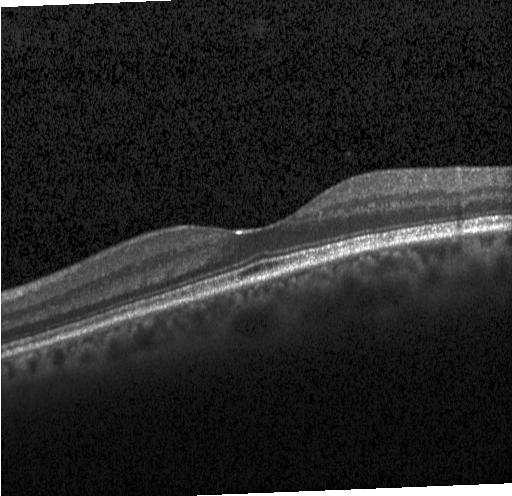

Finding: no choroidal neovascularization, no diabetic macular edema, and no drusen.